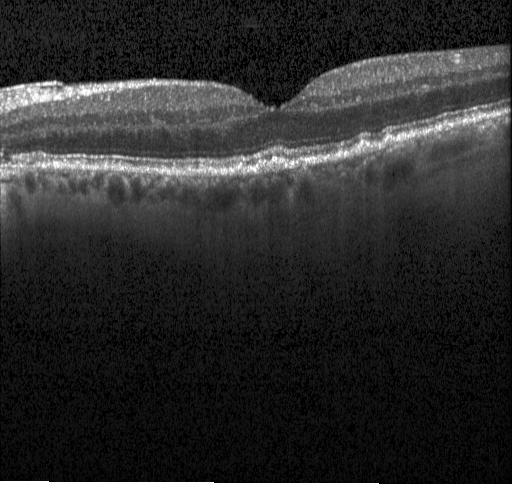

Impression: multiple drusen.